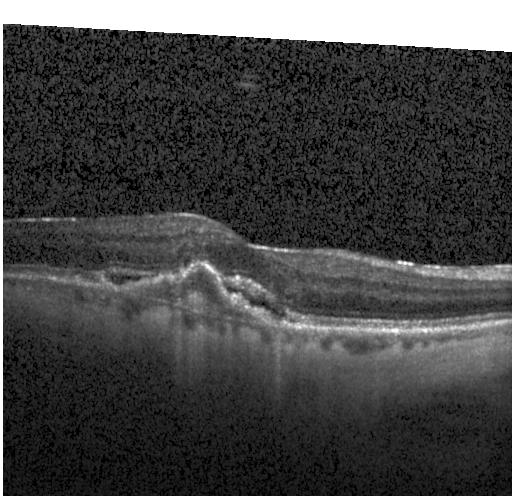 Heidelberg Spectralis; spectral-domain optical coherence tomography; OCT B-scan; macular scan — A choroidal neovascular membrane.